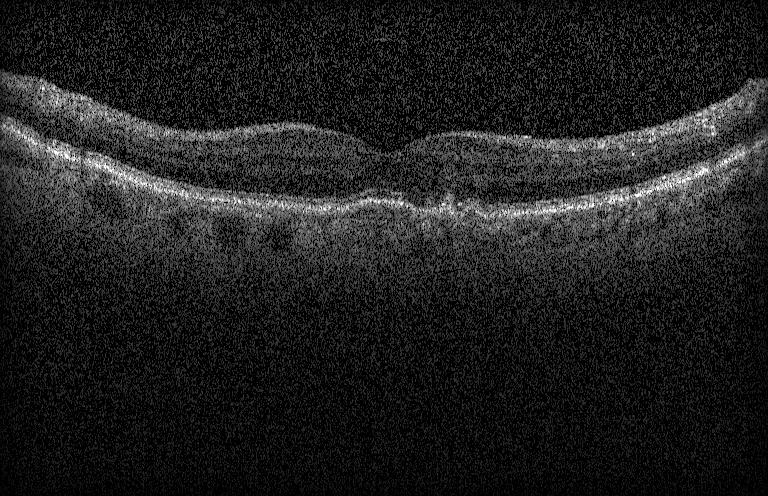

Instrument: Heidelberg Spectralis. Spectral-domain optical coherence tomography. Optical coherence tomography B-scan.
Diagnosis: CNV.